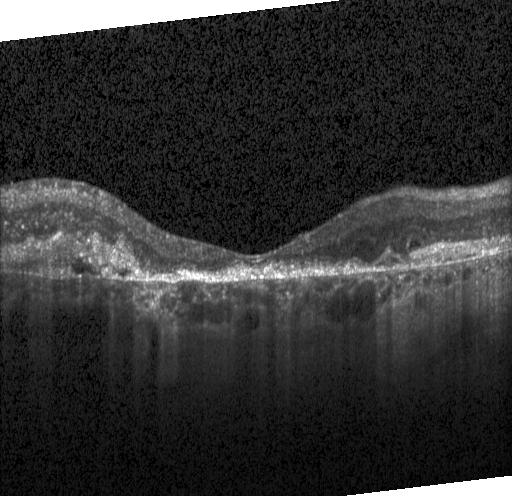
OCT scan showing a choroidal neovascular membrane.